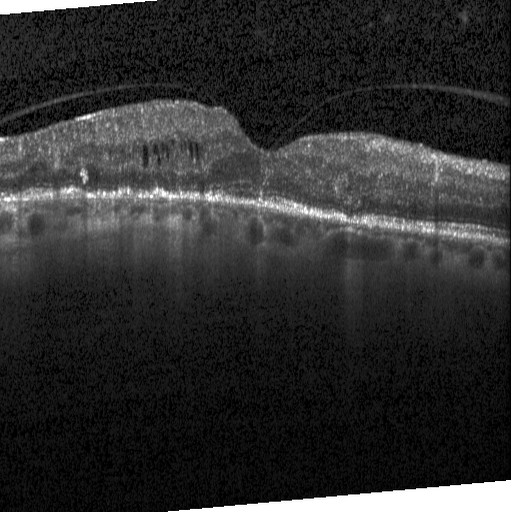
Optical coherence tomography B-scan, macular scan.
The scan shows diabetic macular edema.